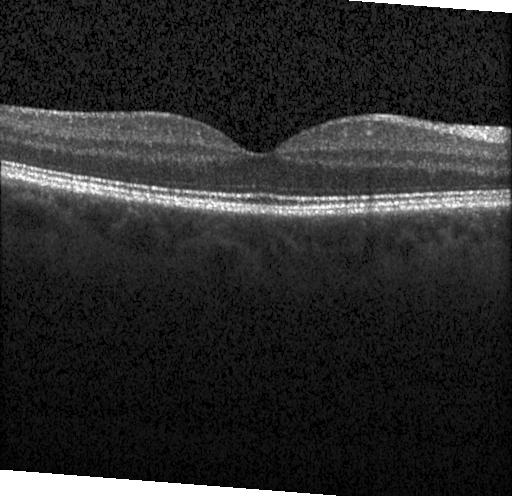 Heidelberg Spectralis OCT system. Centered on the fovea. Spectral-domain optical coherence tomography. OCT line scan — OCT finding: no choroidal neovascularization, diabetic macular edema, or drusen.